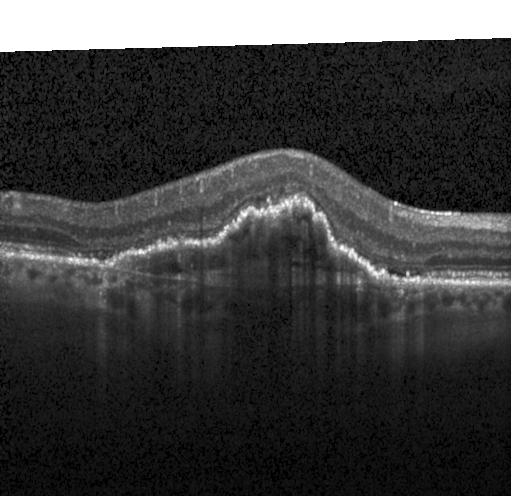
OCT scan showing a choroidal neovascular membrane.